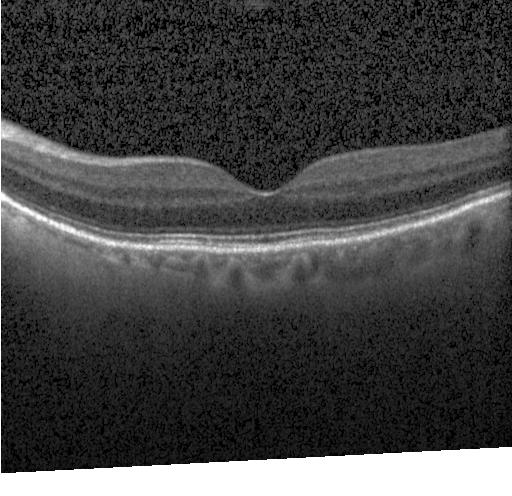
OCT line scan
The scan shows neither choroidal neovascularization, diabetic macular edema, nor drusen.